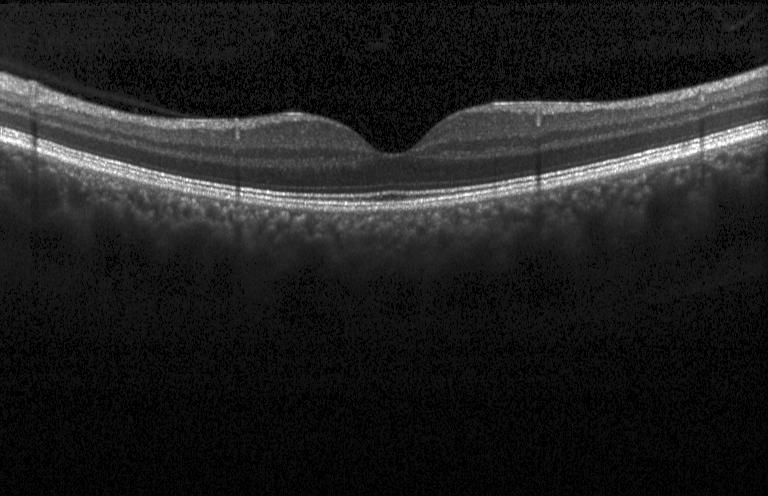

Assessment: no evidence of CNV, DME, or drusen.